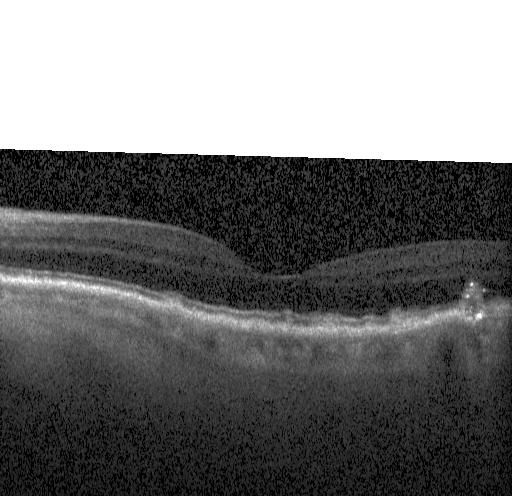

Optical coherence tomography B-scan
Finding: CNV.